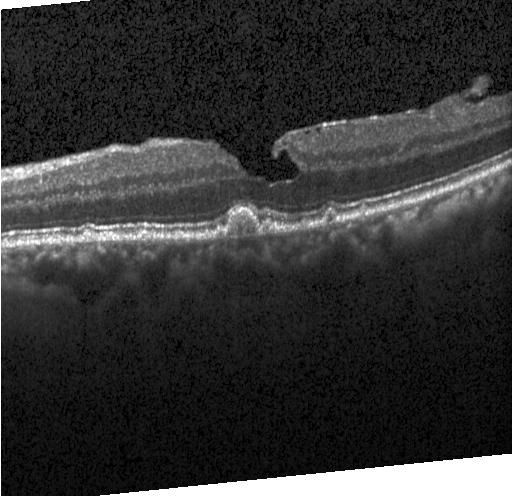

Assessment: drusen.